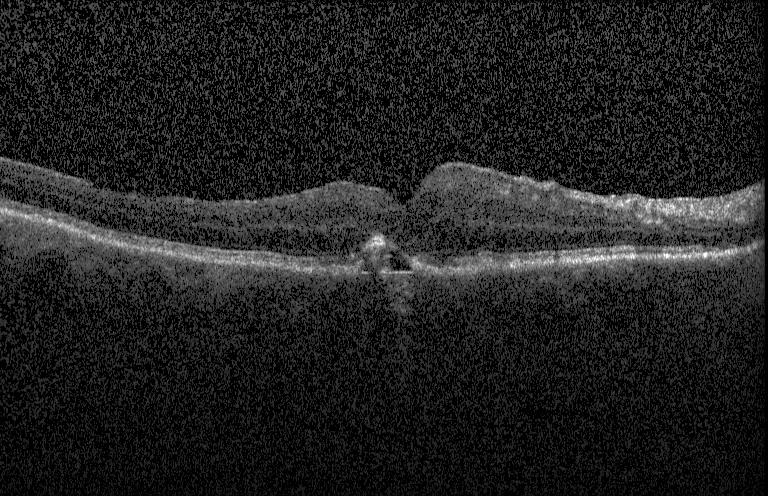
OCT scan showing CNV.